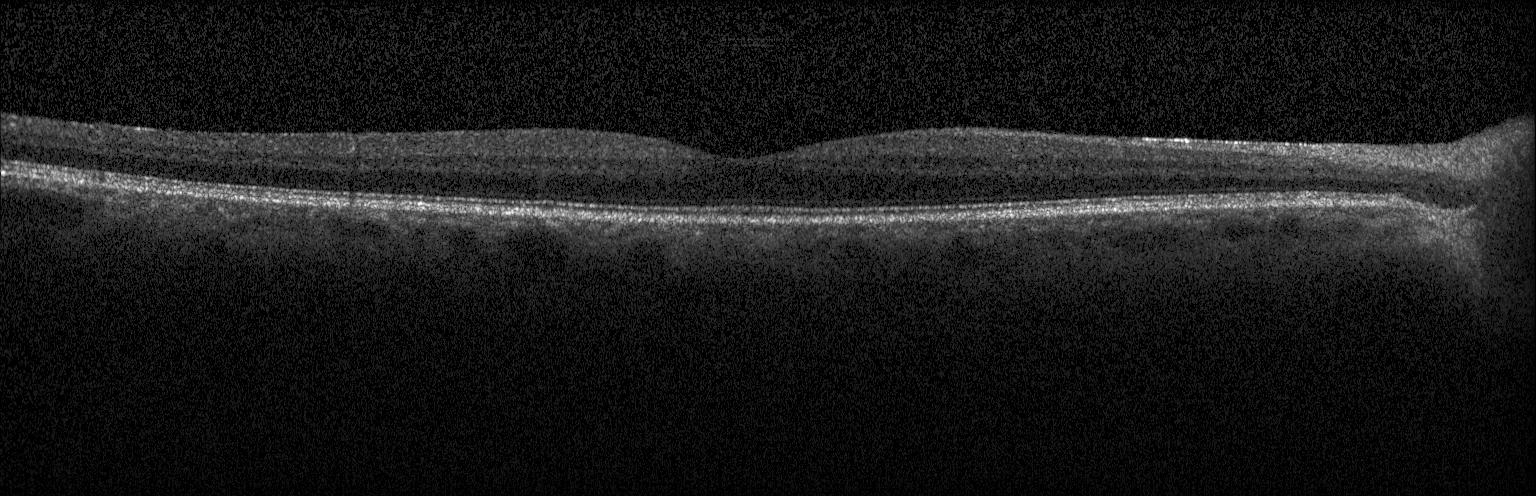
Dx: no evidence of choroidal neovascularization, diabetic macular edema, or drusen.